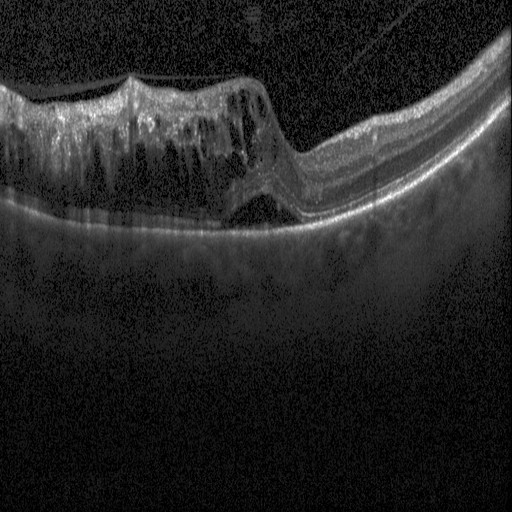

Retinal OCT cross-section showing diabetic macular edema (DME).